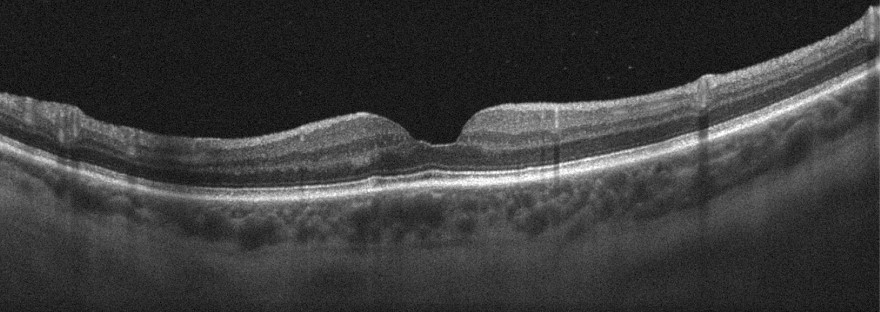
Fovea-centered, Optovue Avanti RTVue XR, optical coherence tomography B-scan.
Dx: age-related macular degeneration.